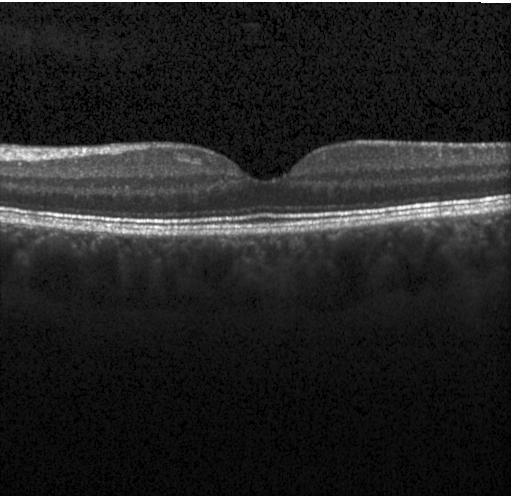
OCT B-scan showing neither CNV, DME, nor drusen.